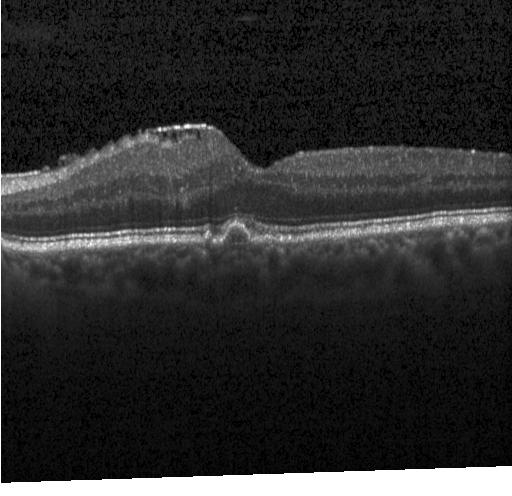 Heidelberg Spectralis, retinal OCT cross-section, fovea-centered, spectral-domain optical coherence tomography. Assessment: drusen.